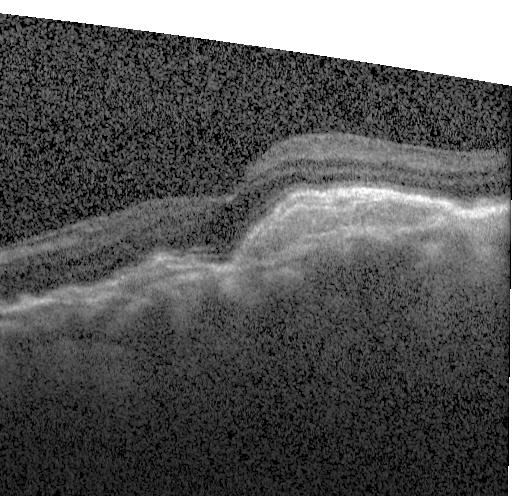 Finding: a choroidal neovascular membrane.